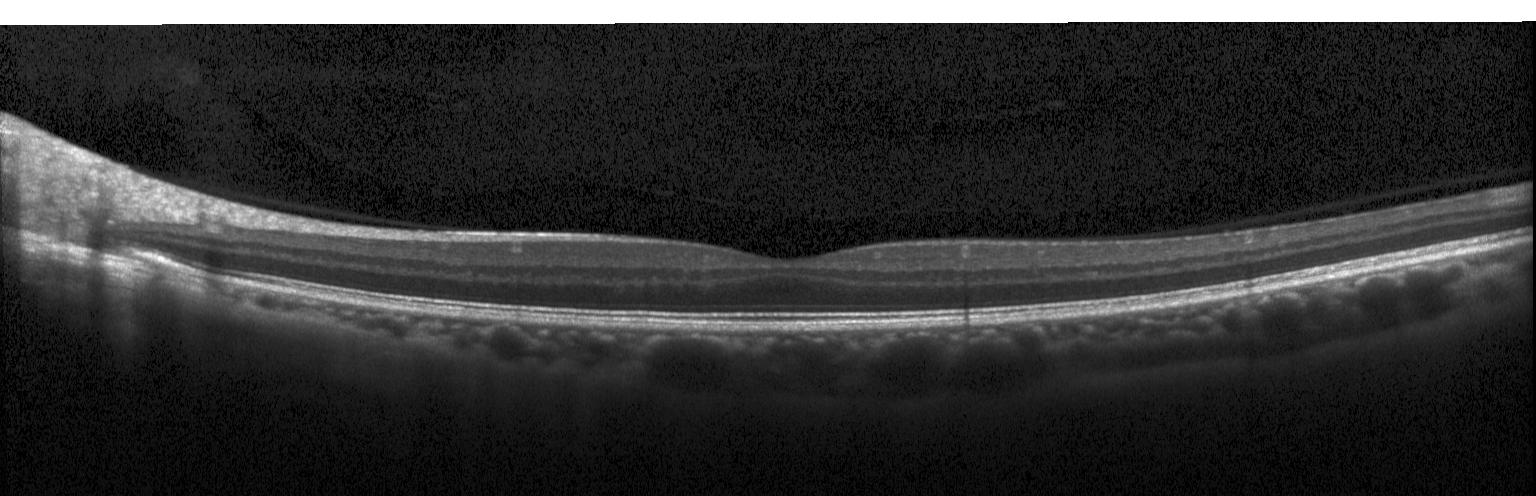
Retinal OCT cross-section showing neither choroidal neovascularization, diabetic macular edema, nor drusen.